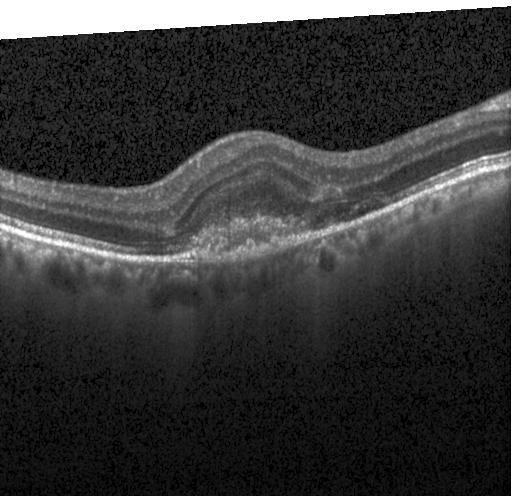

Dx: a choroidal neovascular membrane.